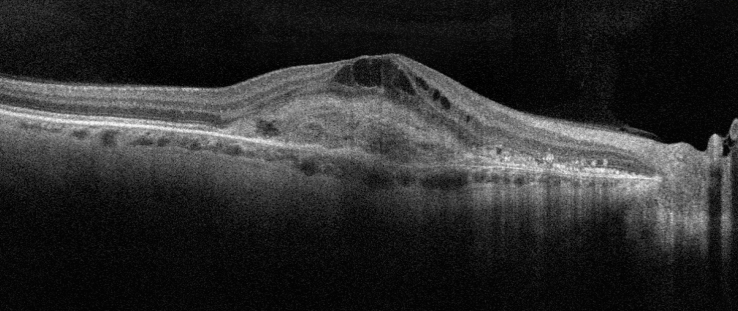 Optovue Avanti RTVue XR. OCT line scan
Diagnosis: age-related macular degeneration.